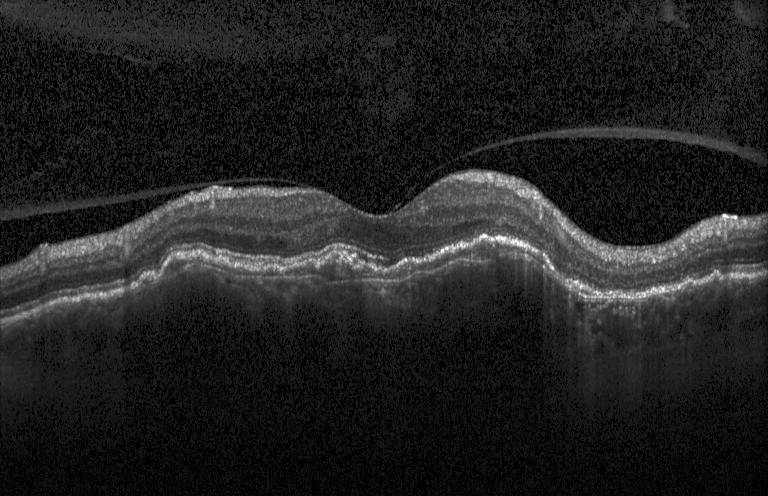
Finding: choroidal neovascularization (CNV).